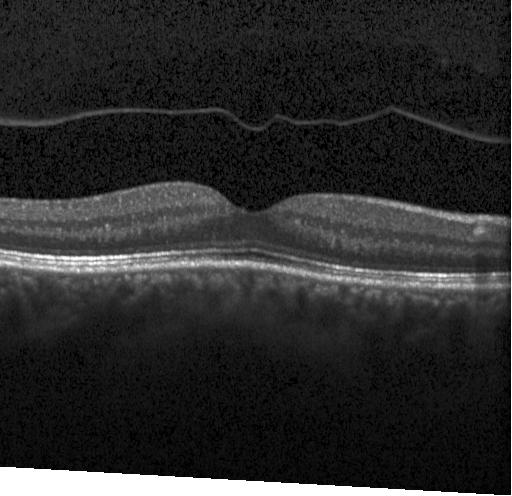
Retinal OCT cross-section, horizontal scan through the fovea — Assessment: no choroidal neovascularization, no diabetic macular edema, and no drusen.